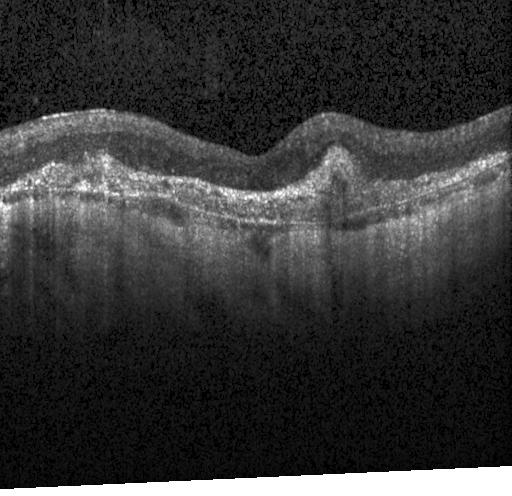
Finding: a choroidal neovascular membrane.